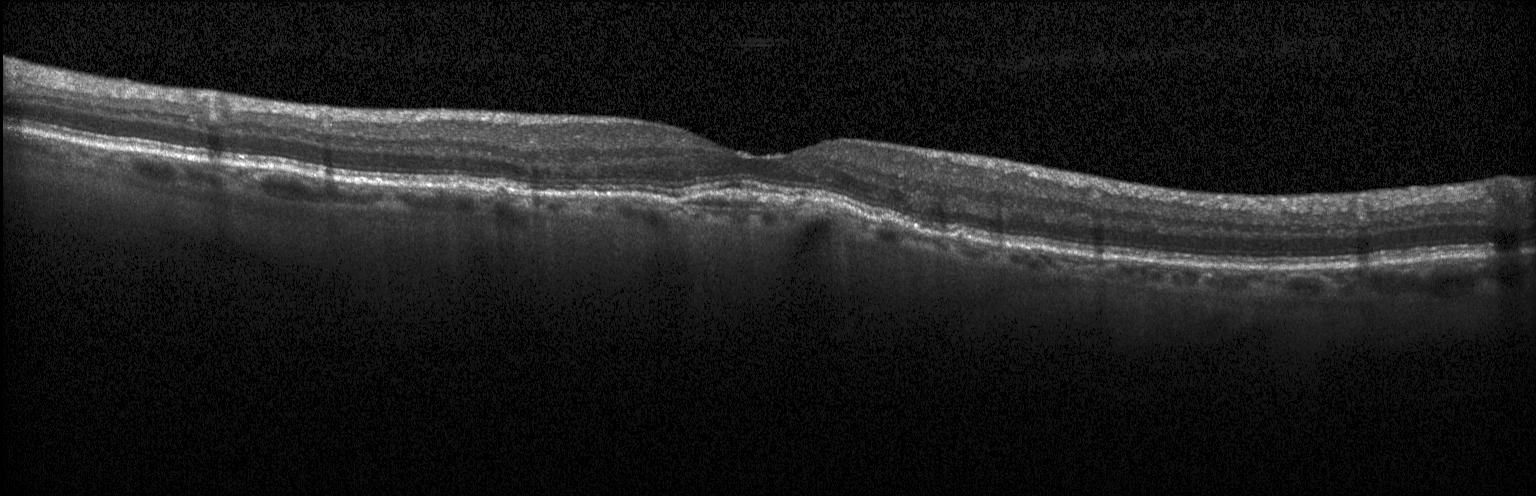 Macular OCT demonstrating a choroidal neovascular membrane.